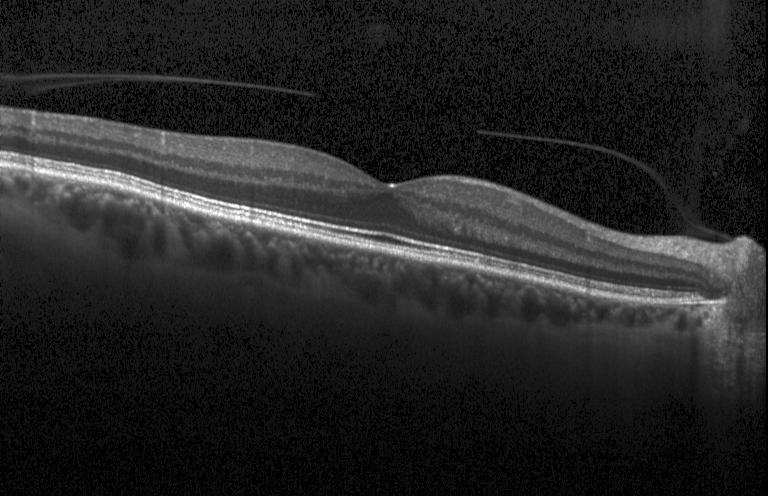

Heidelberg Spectralis, retinal OCT cross-section, through the macula, spectral-domain OCT
Dx: no choroidal neovascularization, diabetic macular edema, or drusen.